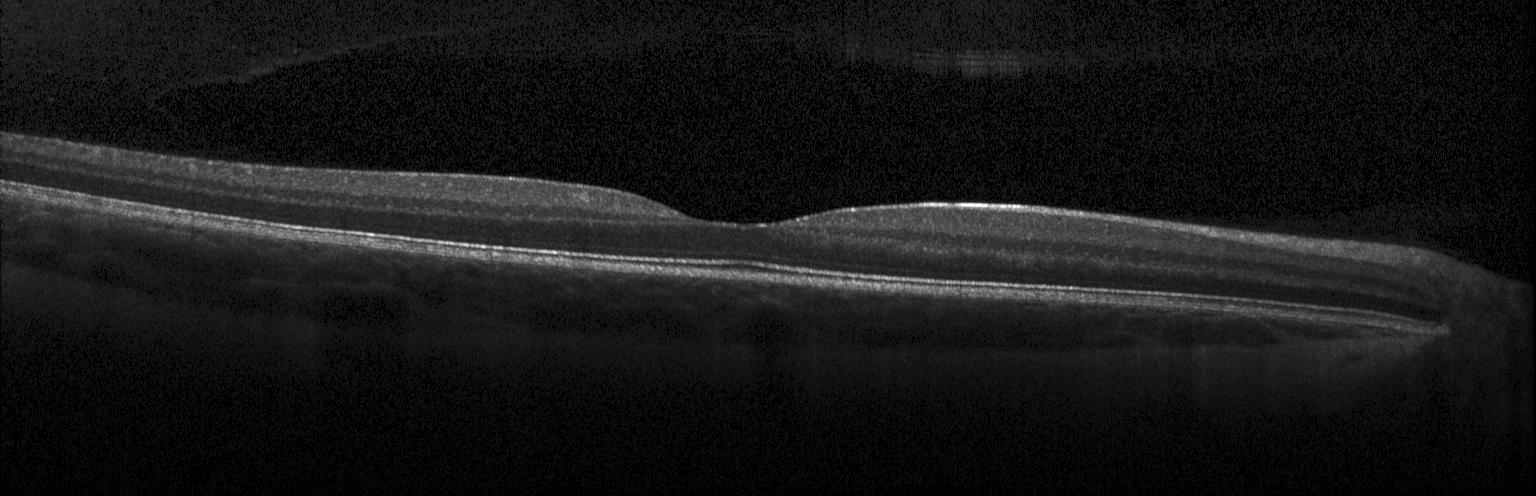 Assessment: no CNV, no DME, and no drusen.